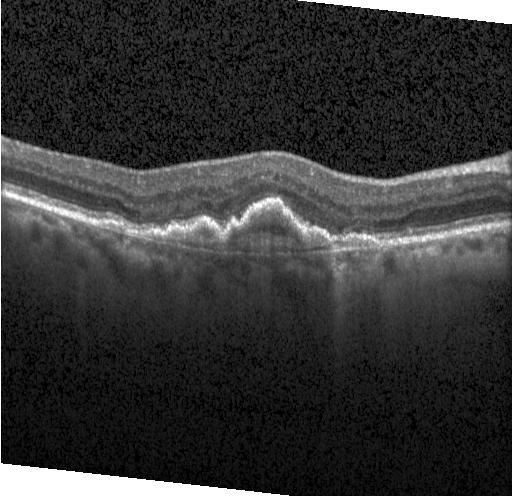

Instrument: Heidelberg Spectralis, OCT B-scan
Diagnosis: CNV.